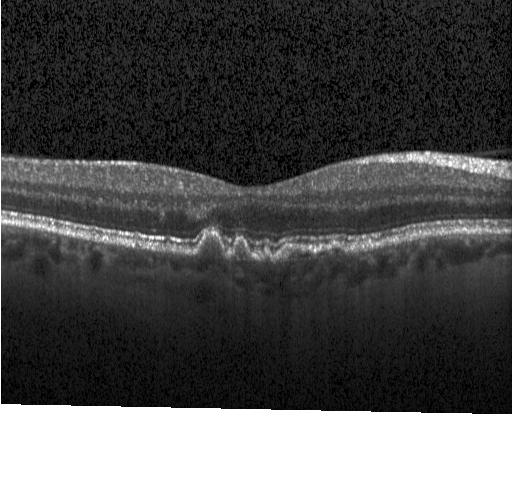

Through the macula. Heidelberg Spectralis OCT system. OCT B-scan.
Sub-RPE drusenoid deposits.